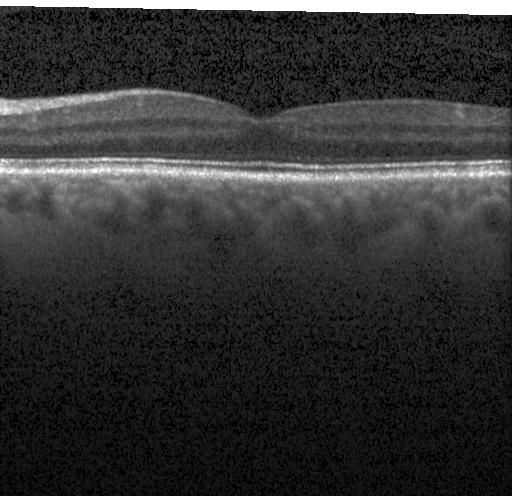 OCT line scan · spectral-domain OCT · Heidelberg Spectralis OCT system. Finding: no choroidal neovascularization, no diabetic macular edema, and no drusen.